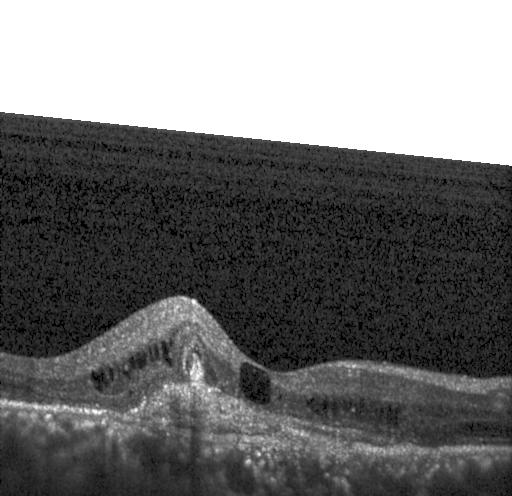 Retinal OCT cross-section, SD-OCT. Finding: a choroidal neovascular membrane.